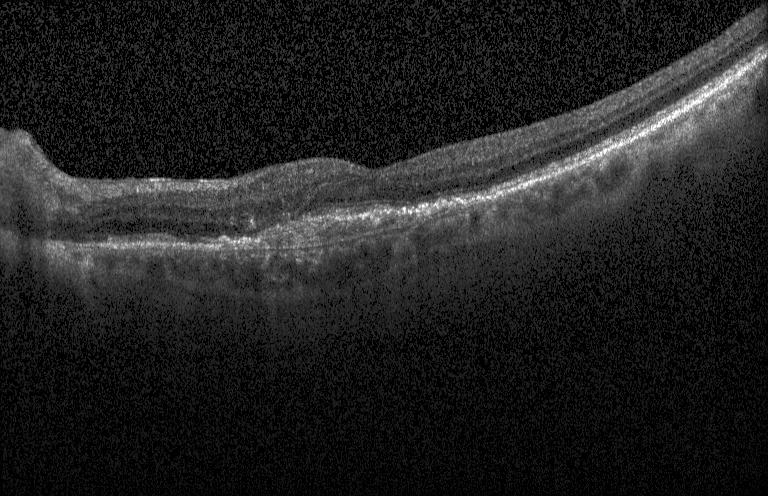 Spectral-domain OCT · Heidelberg Spectralis OCT system · centered on the fovea · retinal OCT cross-section.
This B-scan demonstrates choroidal neovascularization.